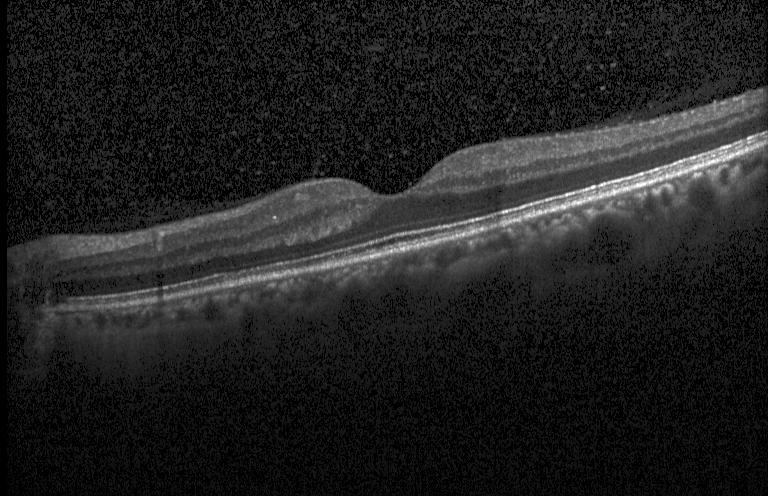
Through the macula, OCT B-scan
Finding: no evidence of choroidal neovascularization, diabetic macular edema, or drusen.